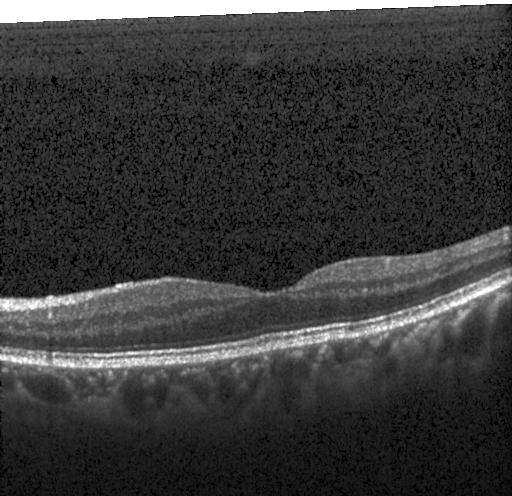
Retinal OCT B-scan
Diagnosis: no choroidal neovascularization, diabetic macular edema, or drusen.